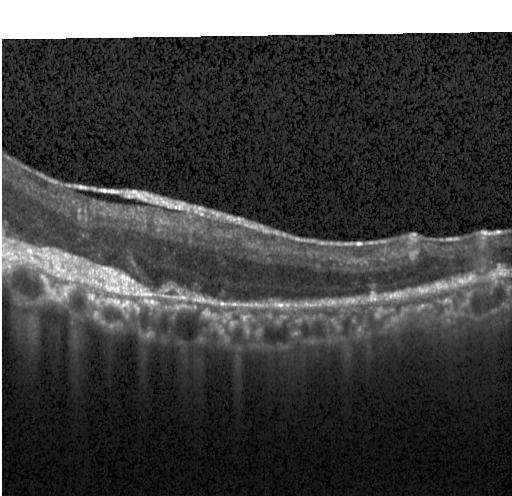
Diagnosis: choroidal neovascularization (CNV).